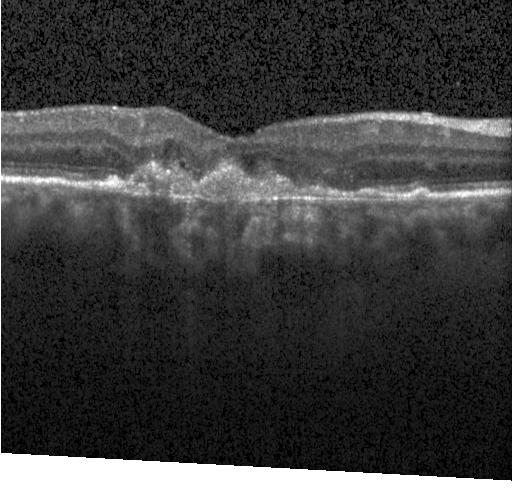 Finding: choroidal neovascularization.